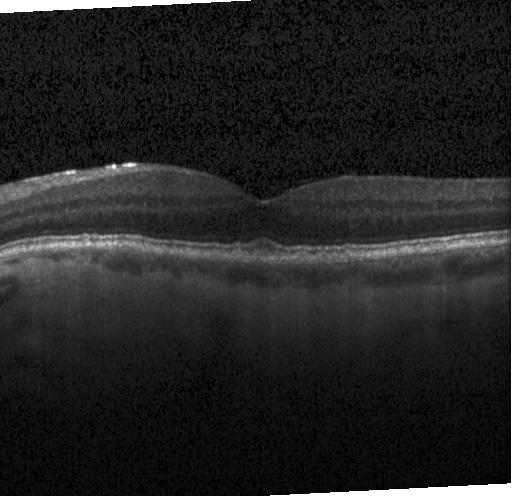
Optical coherence tomography B-scan — This B-scan demonstrates sub-RPE drusenoid deposits.